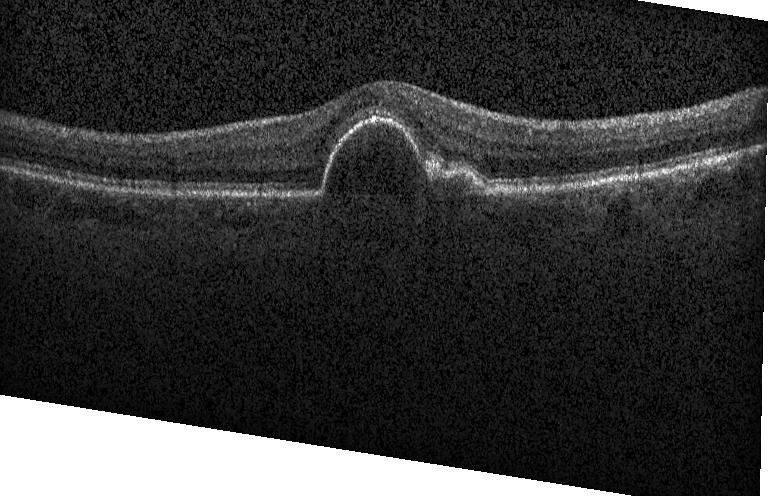
OCT B-scan.
Macular OCT: CNV.